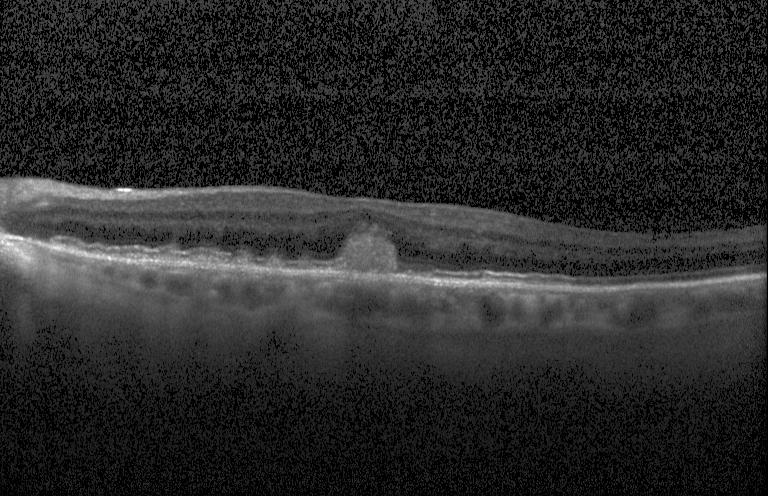
SD-OCT, centered on the fovea, optical coherence tomography scan
This B-scan demonstrates CNV.